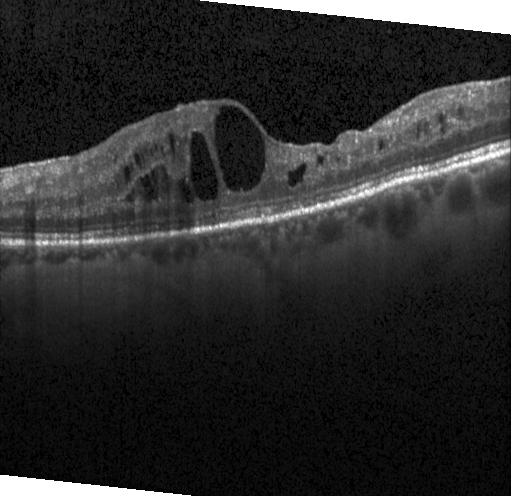 OCT line scan — Finding: diabetic macular edema.